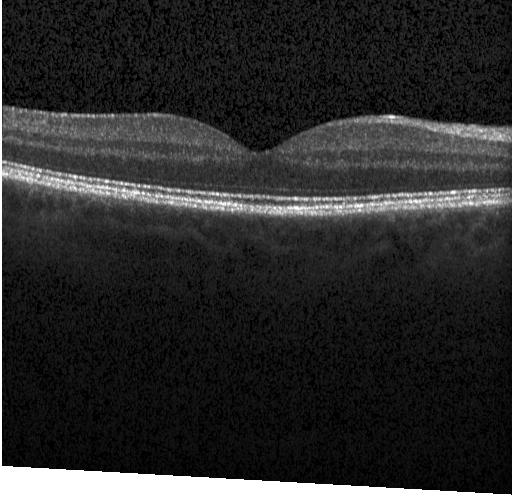 SD-OCT. Heidelberg Spectralis. Retinal OCT B-scan. Through the macula
Assessment: no choroidal neovascularization, no diabetic macular edema, and no drusen.